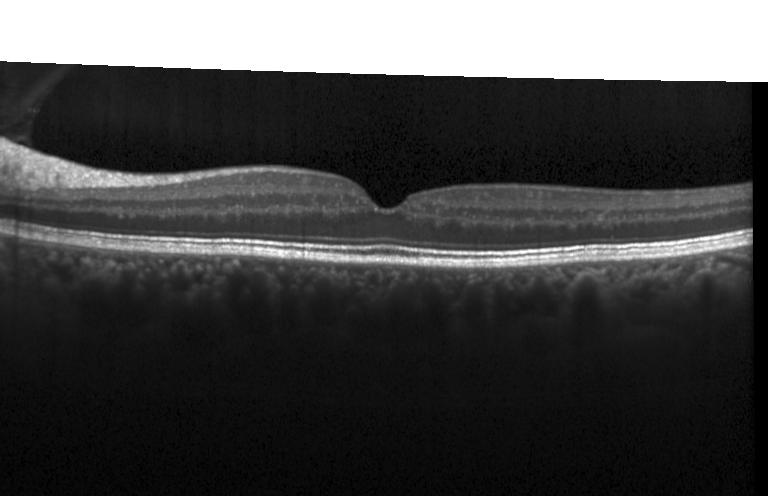
Instrument: Heidelberg Spectralis · macular scan · retinal OCT B-scan · spectral-domain optical coherence tomography — No choroidal neovascularization, no diabetic macular edema, and no drusen.